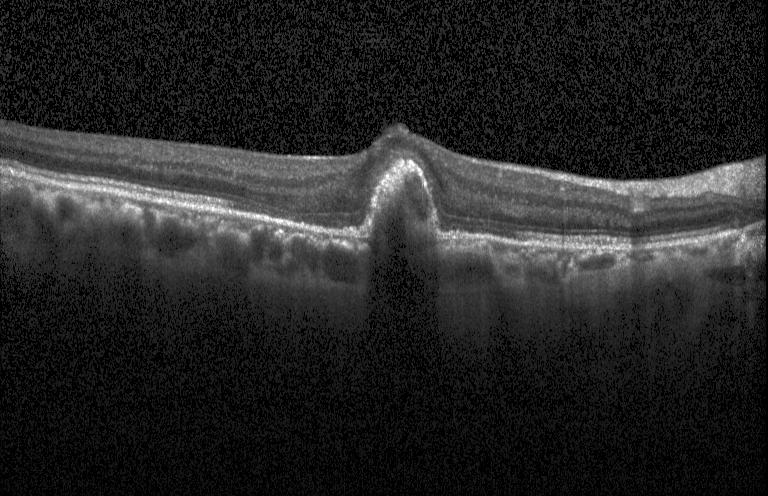
Retinal OCT cross-section showing a choroidal neovascular membrane.